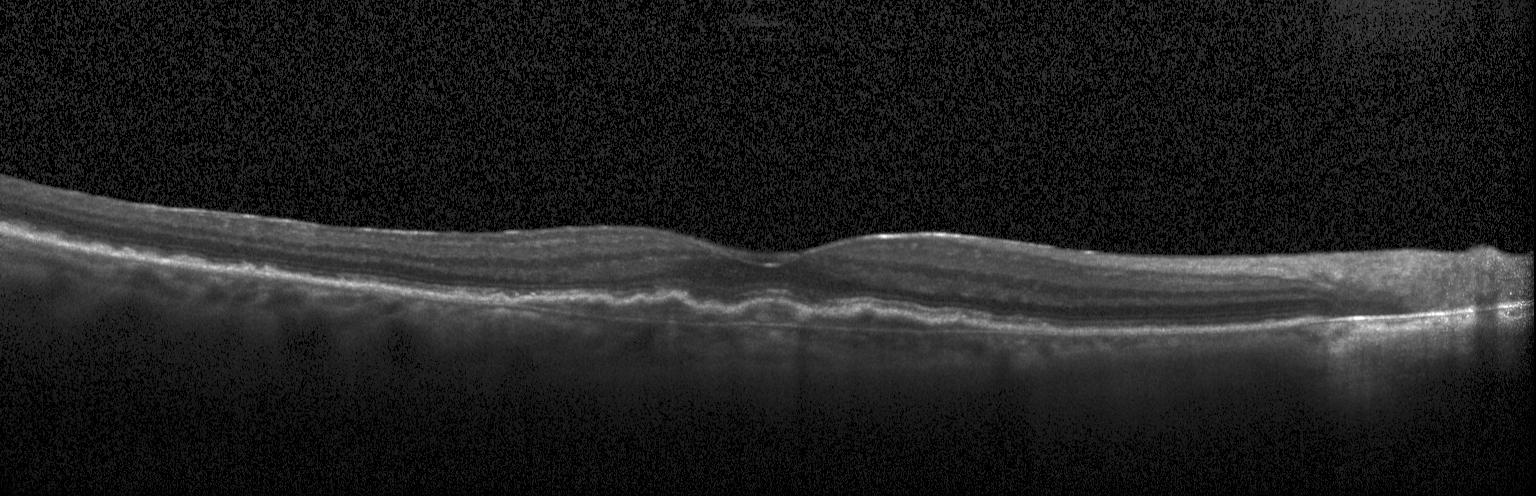 Optical coherence tomography scan — Finding: a choroidal neovascular membrane.